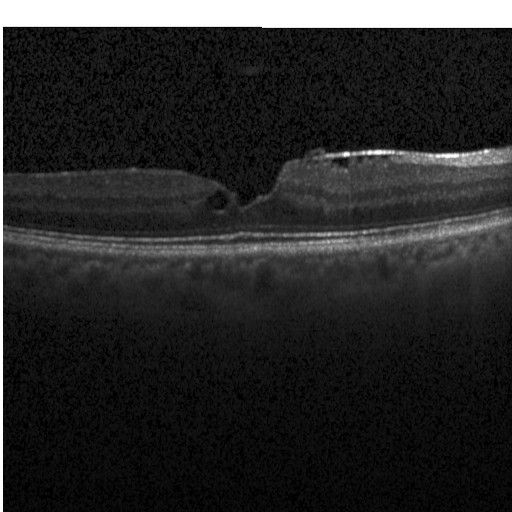

Retinal OCT cross-section showing diabetic macular edema (DME).